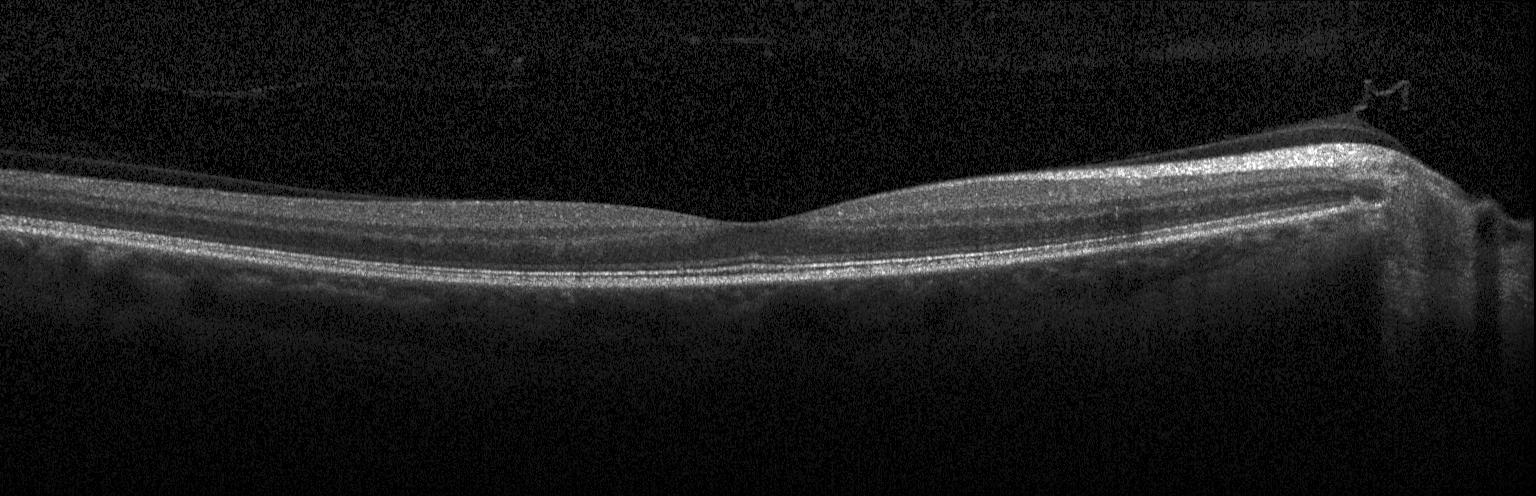

Retinal OCT B-scan, instrument: Heidelberg Spectralis, spectral-domain OCT. The scan shows neither choroidal neovascularization, diabetic macular edema, nor drusen.